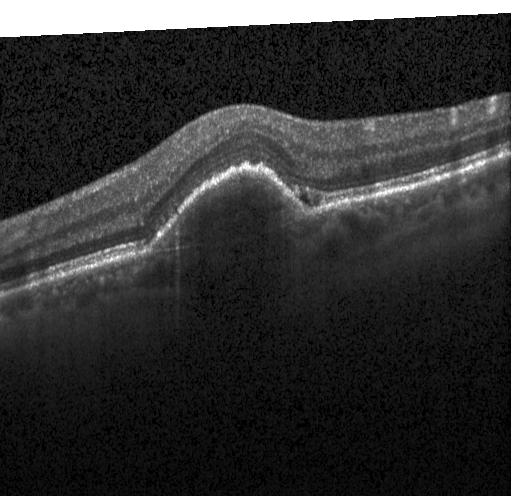
OCT B-scan.
CNV.